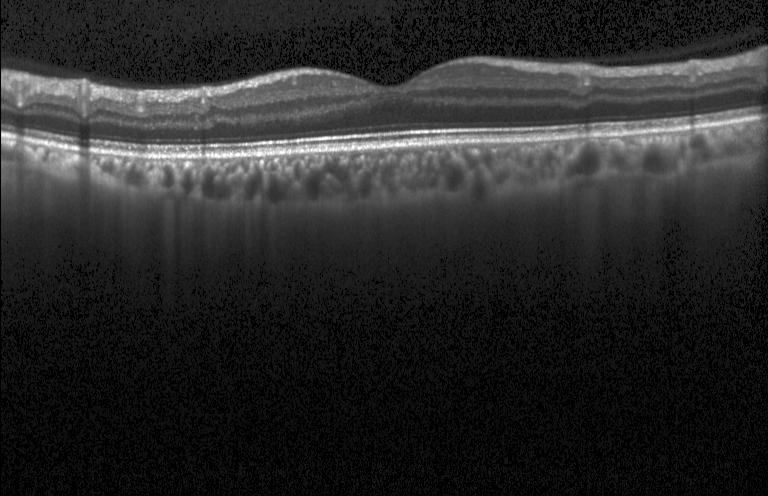
Retinal OCT B-scan; centered on the fovea; Heidelberg Spectralis OCT system; spectral-domain OCT. The scan shows no choroidal neovascularization, no diabetic macular edema, and no drusen.